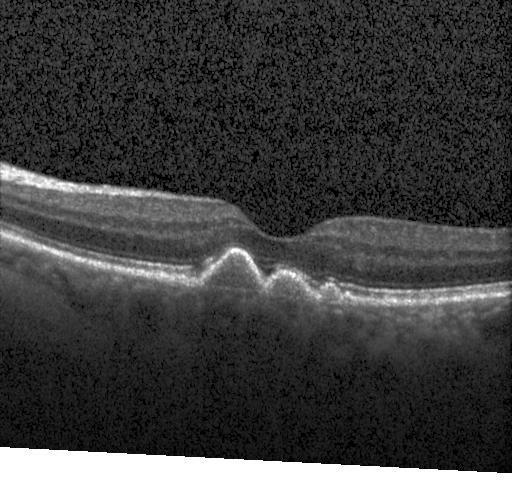
Optical coherence tomography scan.
Multiple drusen.